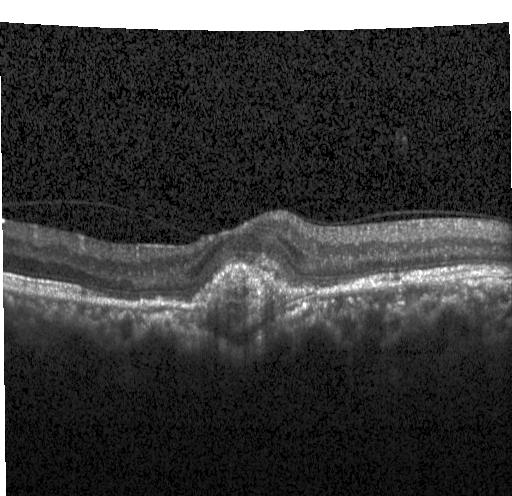
OCT line scan.
A choroidal neovascular membrane.